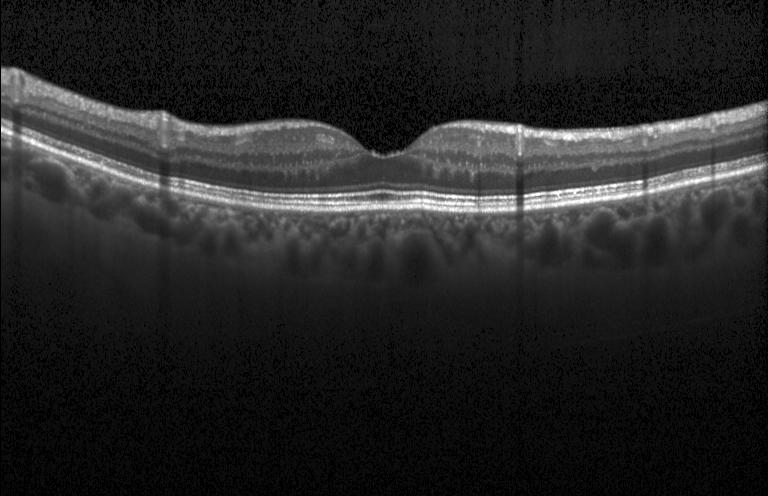 Impression: no evidence of choroidal neovascularization, diabetic macular edema, or drusen.